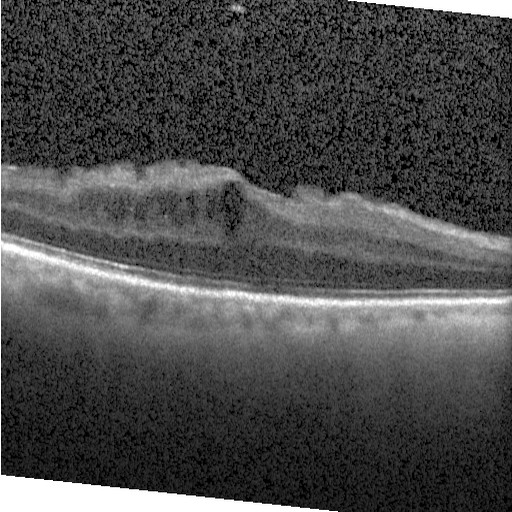
Heidelberg Spectralis. Retinal OCT B-scan. Spectral-domain OCT. Centered on the fovea — Dx: diabetic macular edema.